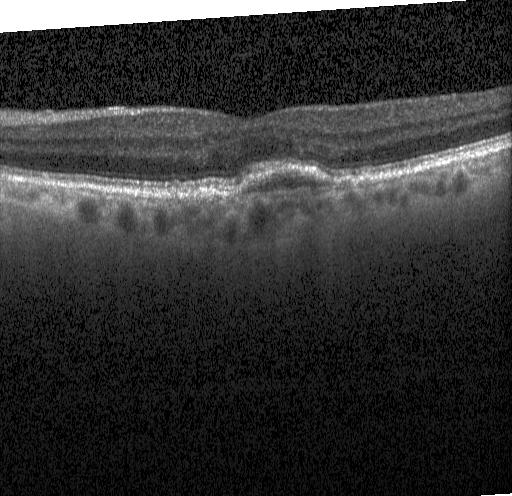

OCT scan showing a choroidal neovascular membrane.